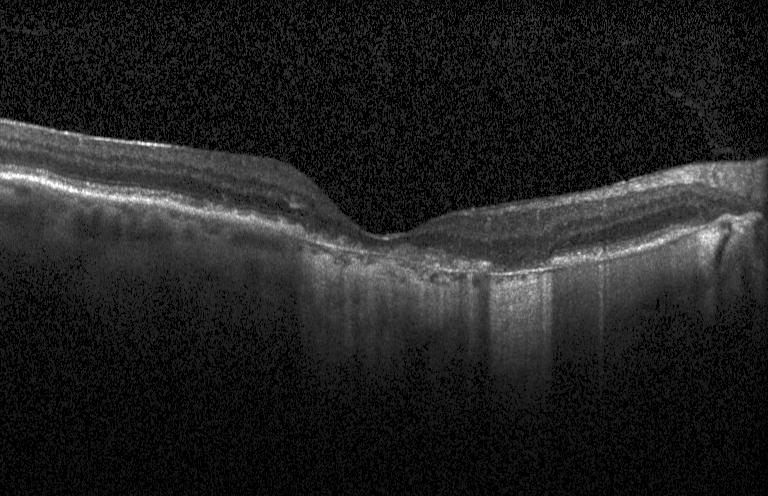 Retinal OCT cross-section; spectral-domain optical coherence tomography; Heidelberg Spectralis. Choroidal neovascularization (CNV).